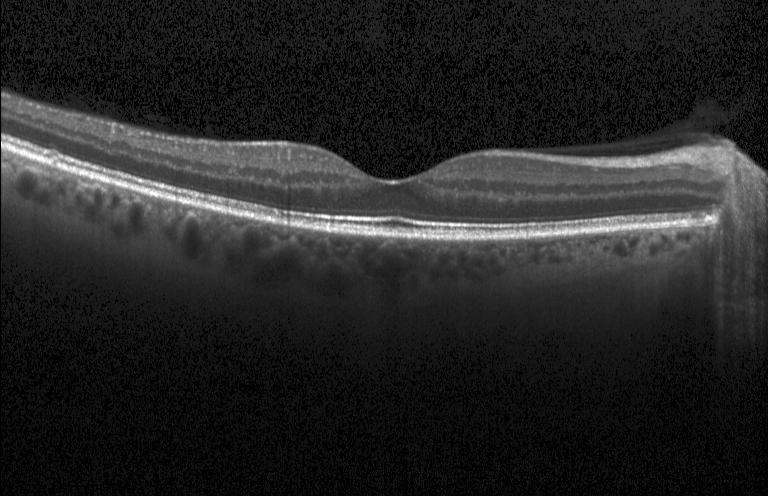
Instrument: Heidelberg Spectralis · SD-OCT · optical coherence tomography B-scan · macular scan — Assessment: neither choroidal neovascularization, diabetic macular edema, nor drusen.